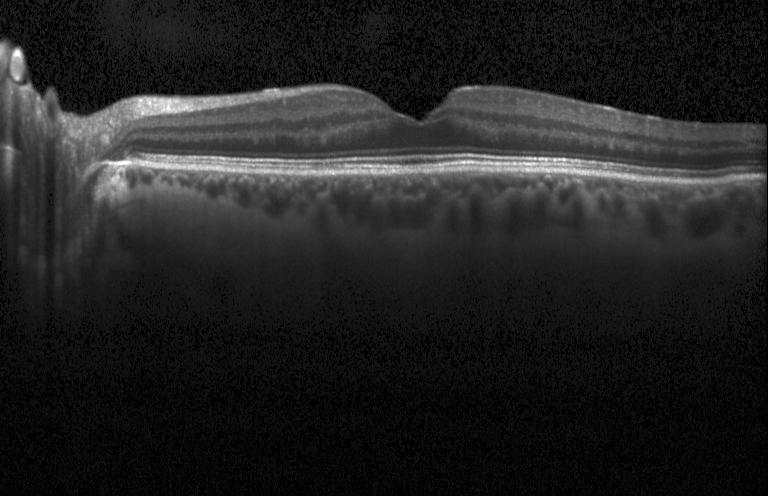 Impression: no choroidal neovascularization, diabetic macular edema, or drusen.